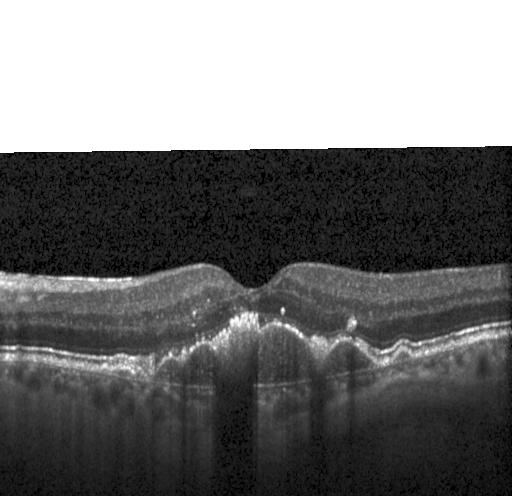

Retinal OCT cross-section, spectral-domain optical coherence tomography, fovea-centered
Assessment: choroidal neovascularization (CNV).